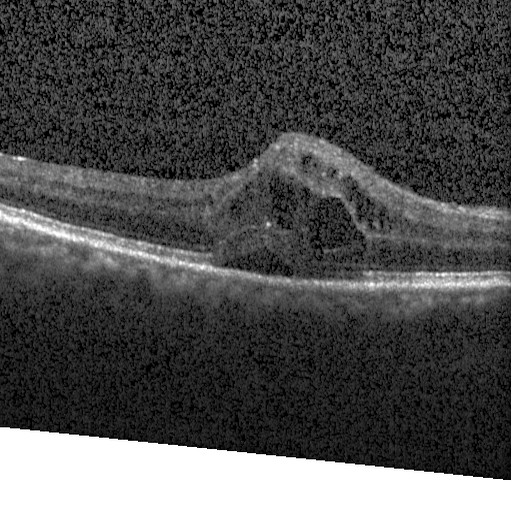
The scan shows diabetic macular edema (DME).